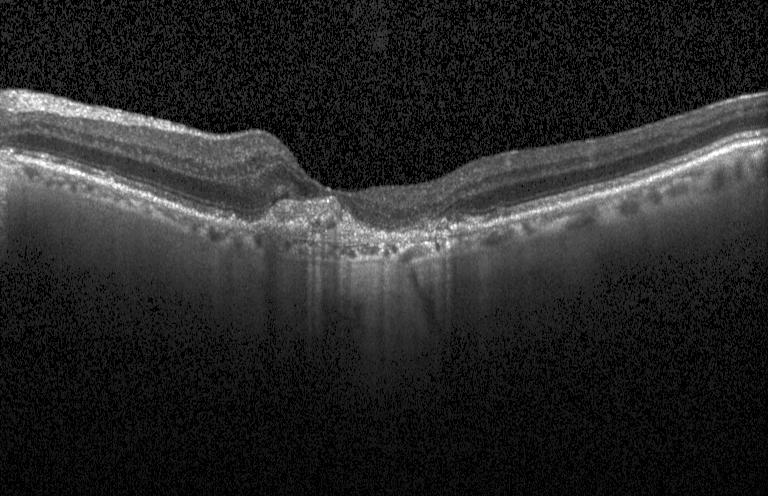

Finding: a choroidal neovascular membrane.